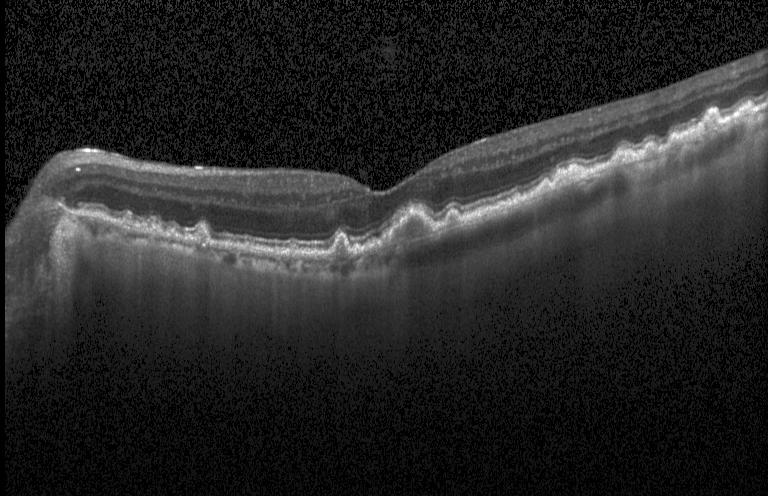

Multiple drusen.